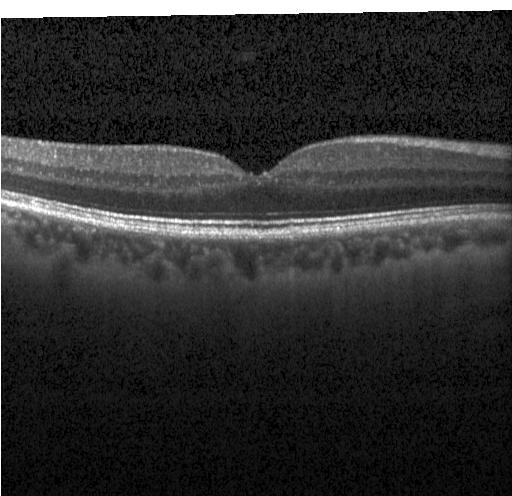

Heidelberg Spectralis OCT system. Spectral-domain OCT. OCT B-scan
Impression: no choroidal neovascularization, no diabetic macular edema, and no drusen.